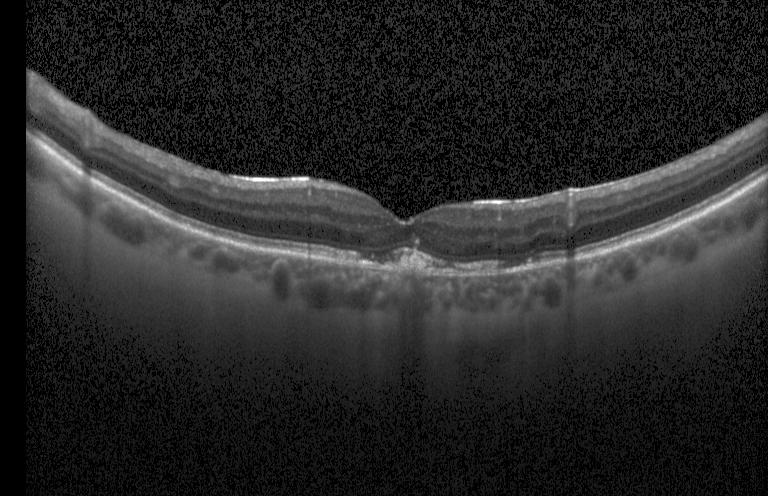
Through the macula; spectral-domain optical coherence tomography; optical coherence tomography B-scan; Heidelberg Spectralis OCT system. The scan shows a choroidal neovascular membrane.